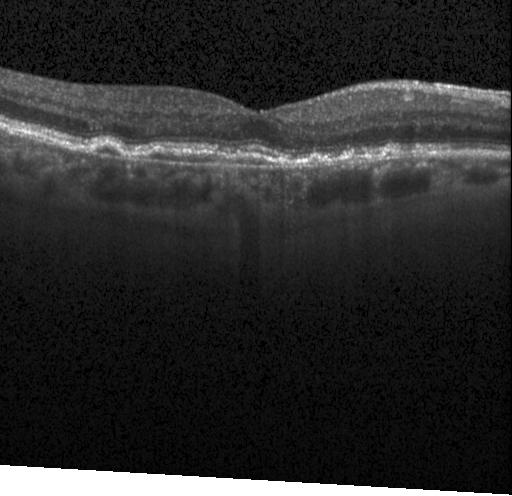

The scan shows a choroidal neovascular membrane.